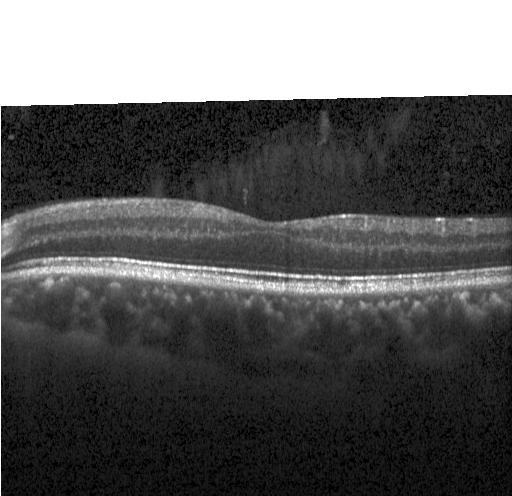
Optical coherence tomography scan
The scan shows no CNV, no DME, and no drusen.